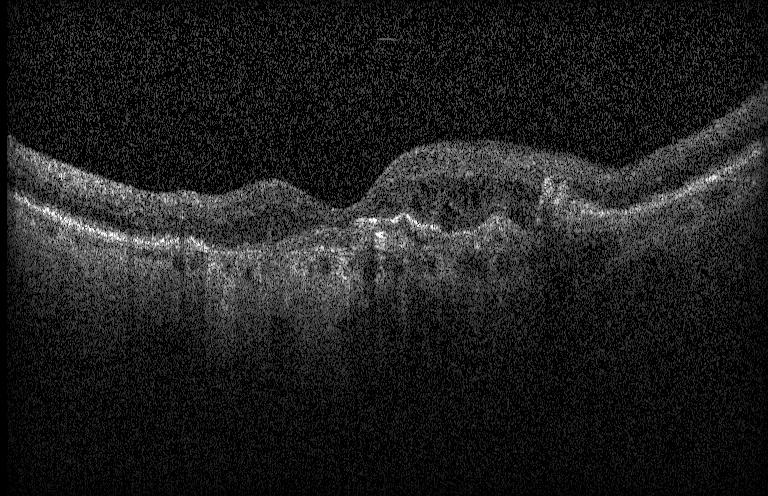

OCT finding: a choroidal neovascular membrane.